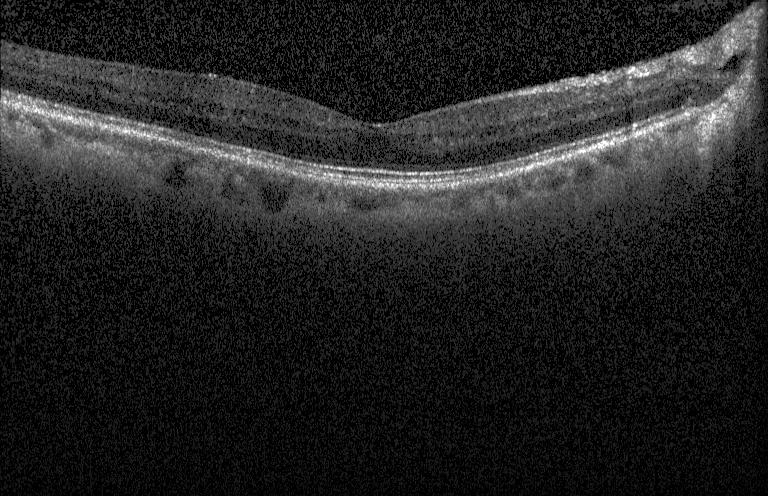 Horizontal scan through the fovea, retinal OCT B-scan, acquired on a Heidelberg Spectralis, SD-OCT
Assessment: no choroidal neovascularization, no diabetic macular edema, and no drusen.